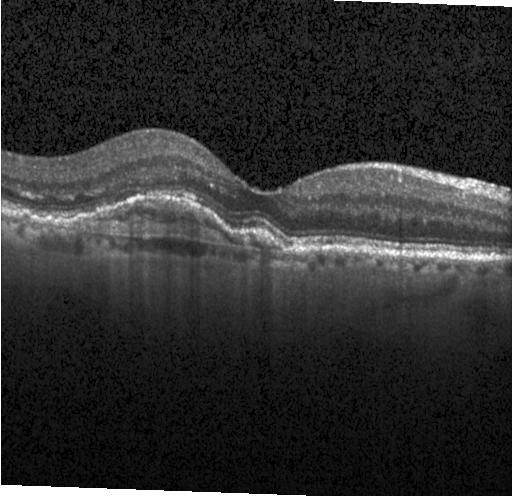
Diagnosis: a choroidal neovascular membrane.